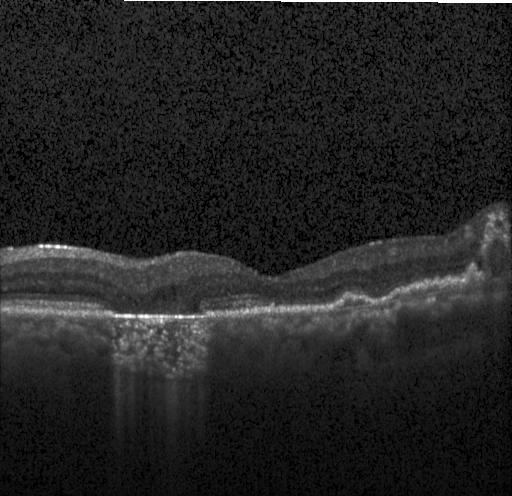 OCT line scan; SD-OCT; Heidelberg Spectralis OCT system. Dx: a choroidal neovascular membrane.